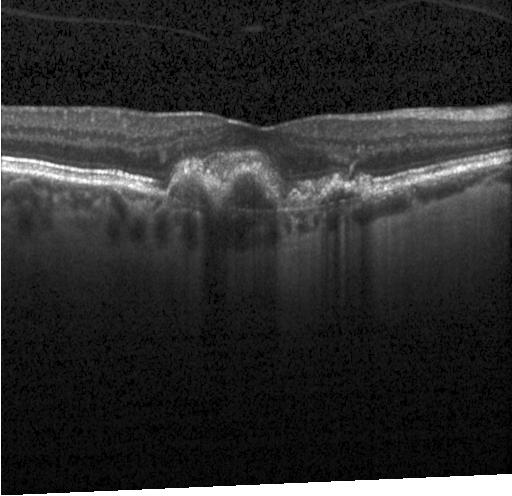
Impression: choroidal neovascularization.